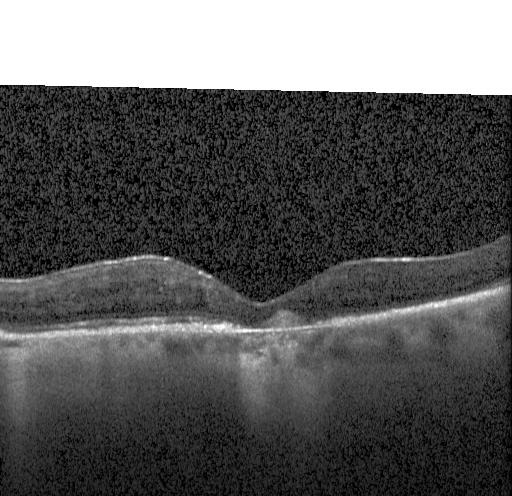 SD-OCT. Heidelberg Spectralis OCT system. Through the macula. OCT line scan. OCT finding: CNV.